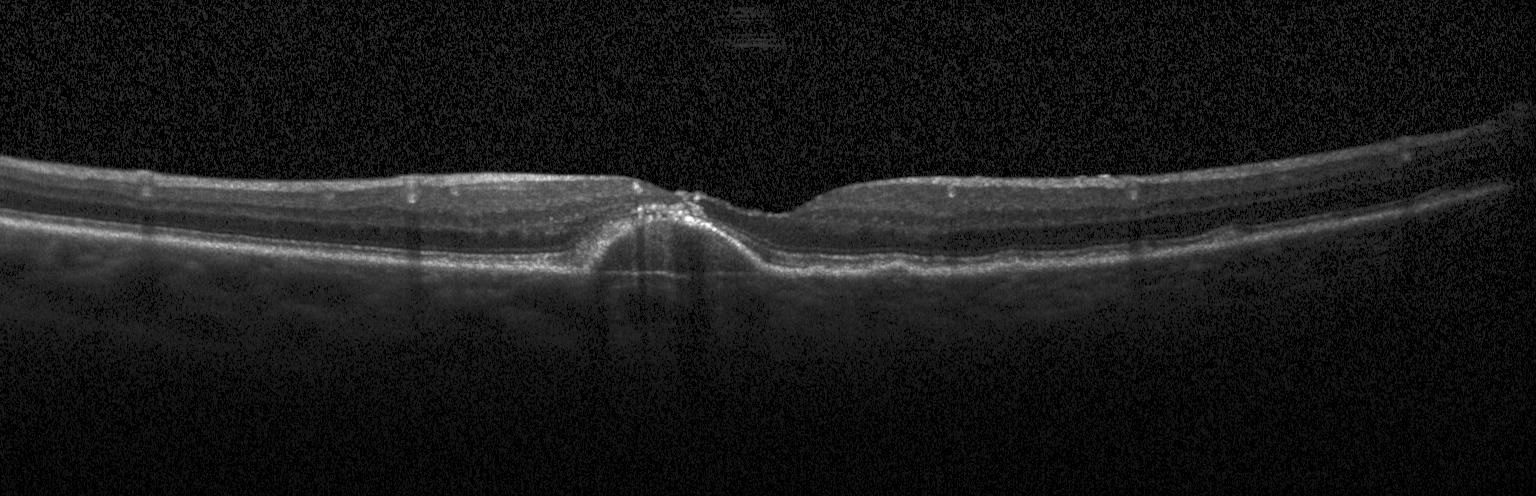
Retinal OCT cross-section showing a choroidal neovascular membrane.